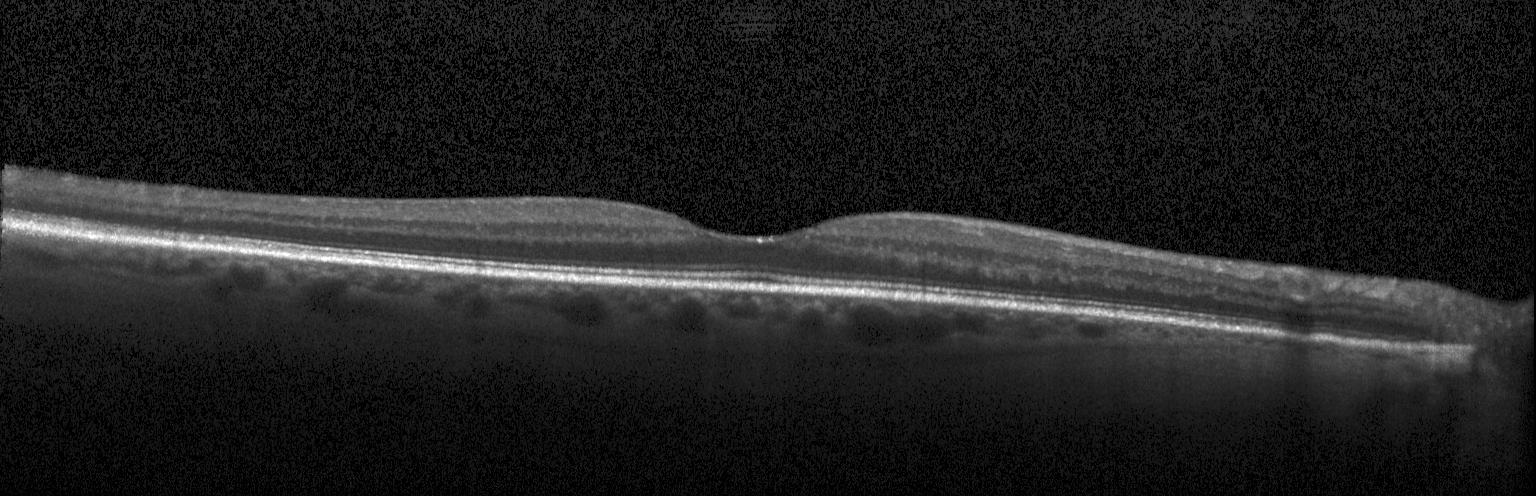
Spectral-domain optical coherence tomography; Heidelberg Spectralis; through the macula; OCT B-scan — Diagnosis: no evidence of choroidal neovascularization, diabetic macular edema, or drusen.